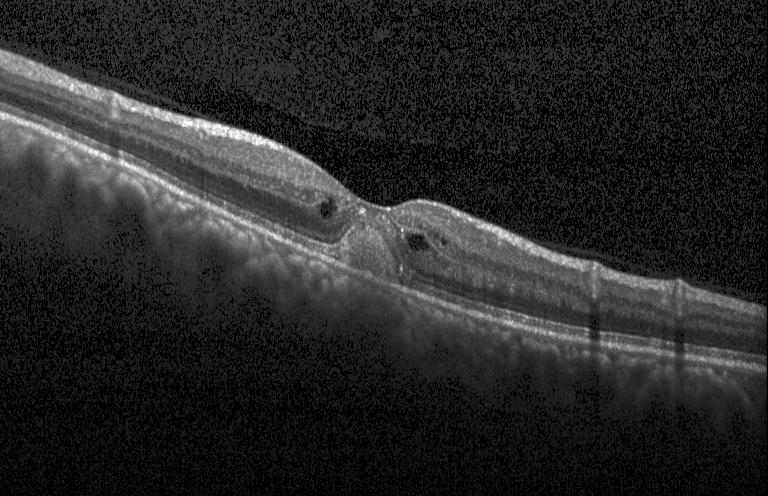 Spectral-domain optical coherence tomography, optical coherence tomography scan — Diagnosis: choroidal neovascularization (CNV).